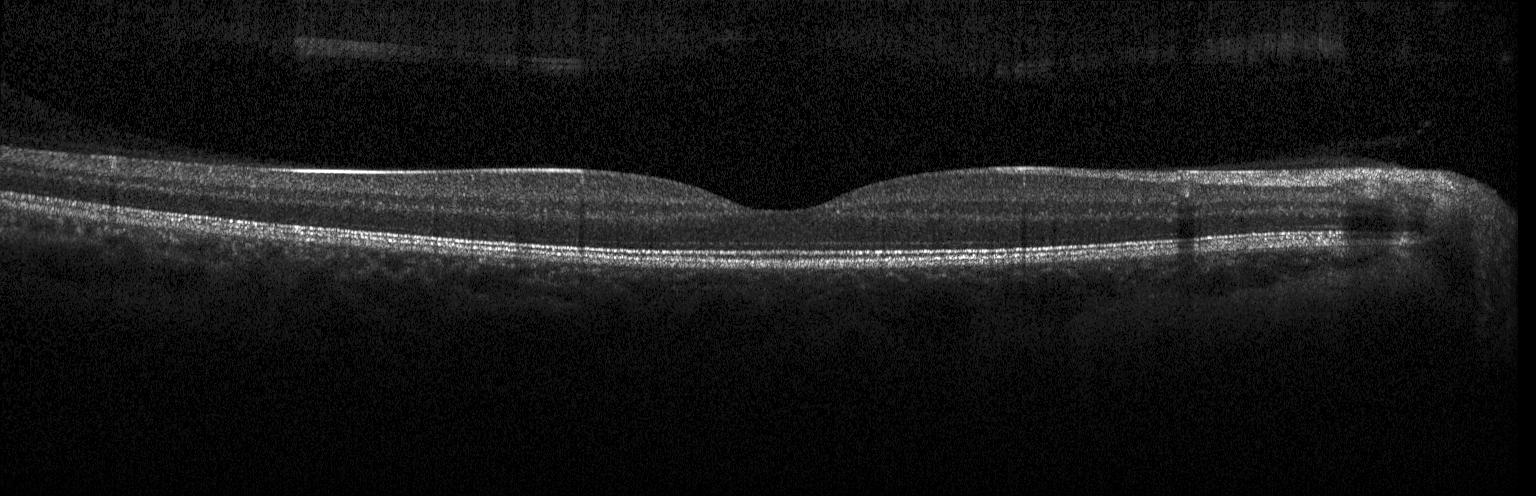 Dx: no choroidal neovascularization, no diabetic macular edema, and no drusen.